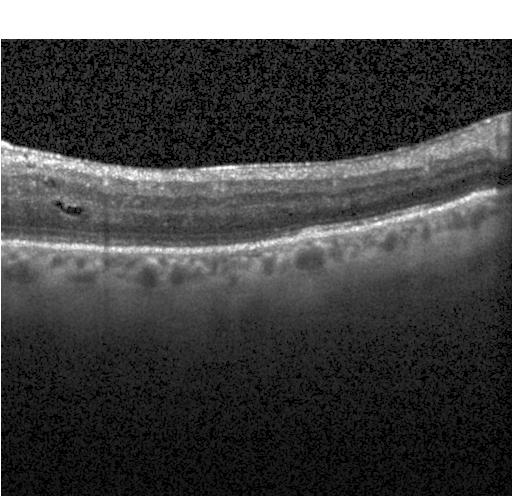 OCT B-scan · horizontal scan through the fovea
Macular OCT: diabetic macular edema (DME).